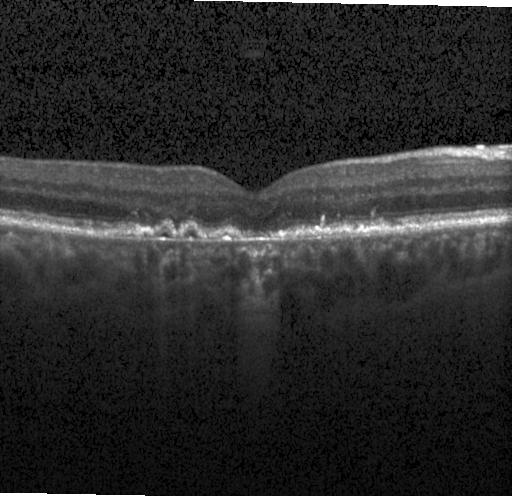
Impression: CNV.